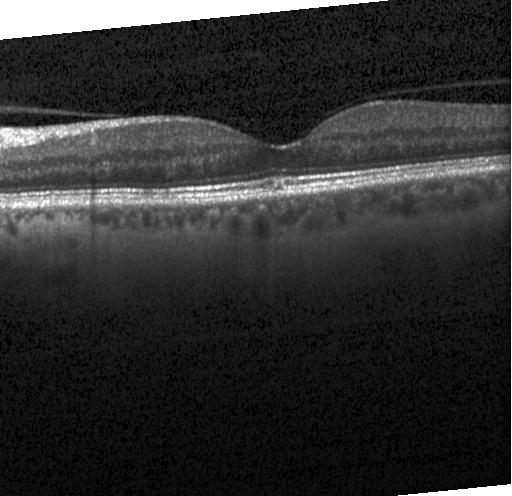 Macular OCT: no CNV, no DME, and no drusen.